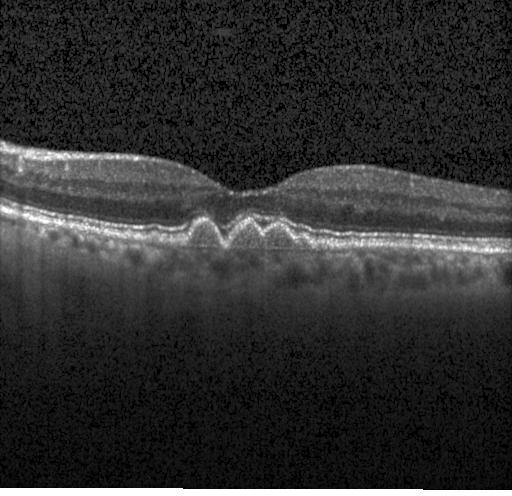
Spectral-domain OCT, OCT B-scan, through the macula, Heidelberg Spectralis OCT system
OCT finding: sub-RPE drusenoid deposits.